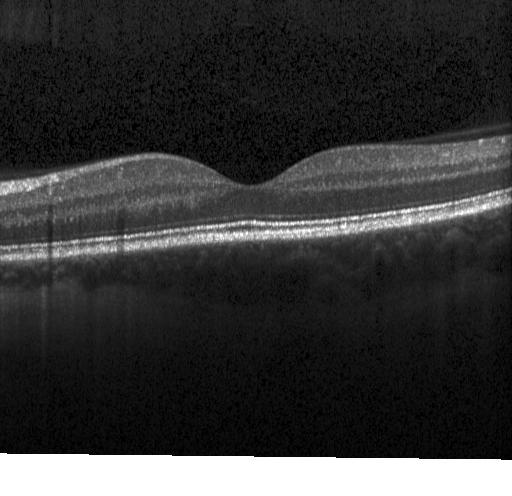
Macular OCT demonstrating no choroidal neovascularization, no diabetic macular edema, and no drusen.